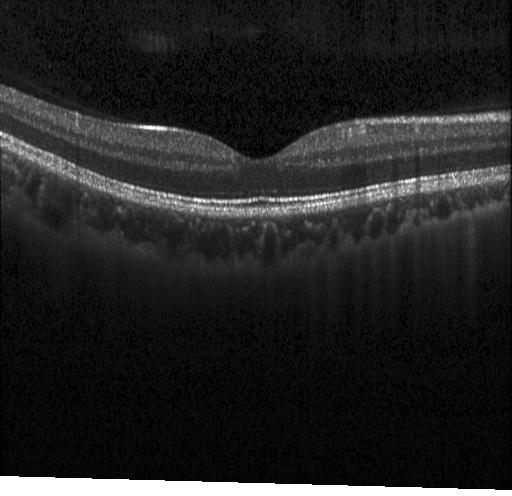

Instrument: Heidelberg Spectralis; spectral-domain OCT; through the macula; OCT B-scan
No evidence of choroidal neovascularization, diabetic macular edema, or drusen.